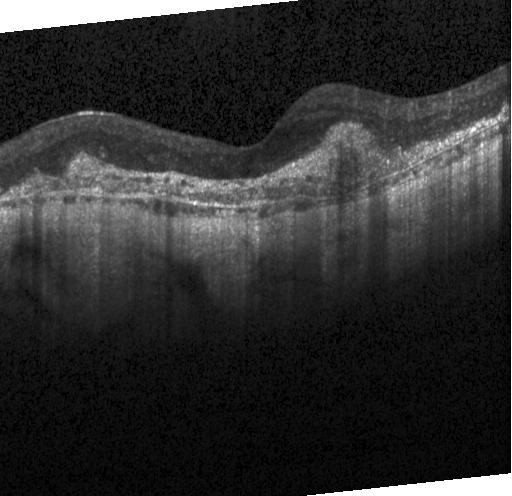 Fovea-centered · retinal OCT B-scan.
Finding: choroidal neovascularization (CNV).